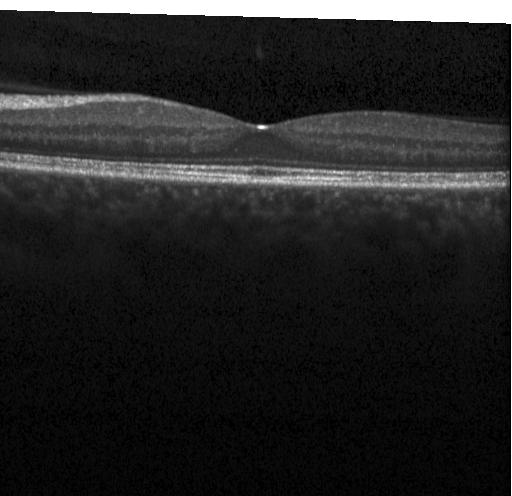 Horizontal scan through the fovea · spectral-domain OCT · optical coherence tomography scan. Impression: no evidence of CNV, DME, or drusen.